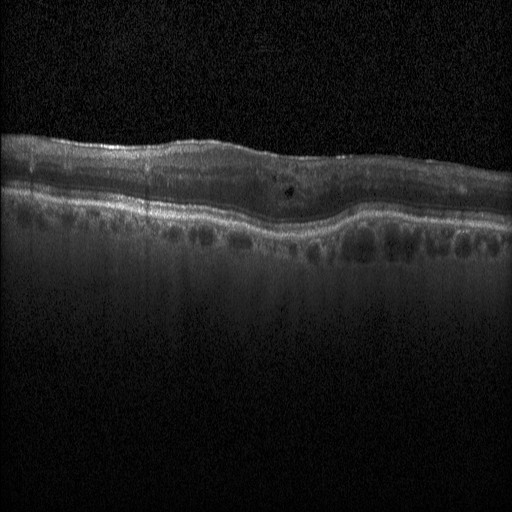

Optical coherence tomography scan — Diagnosis: DME.